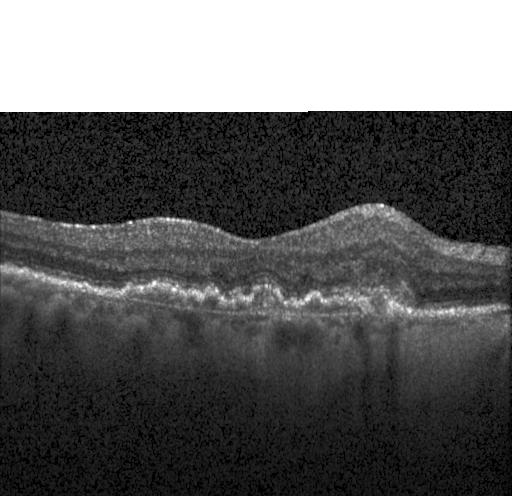 Diagnosis: CNV.